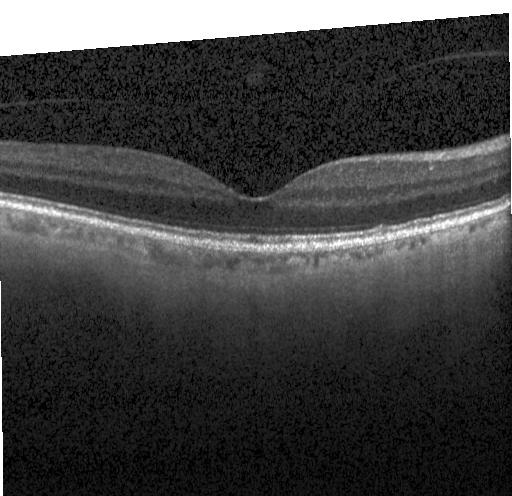 Retinal OCT cross-section showing no choroidal neovascularization, no diabetic macular edema, and no drusen.